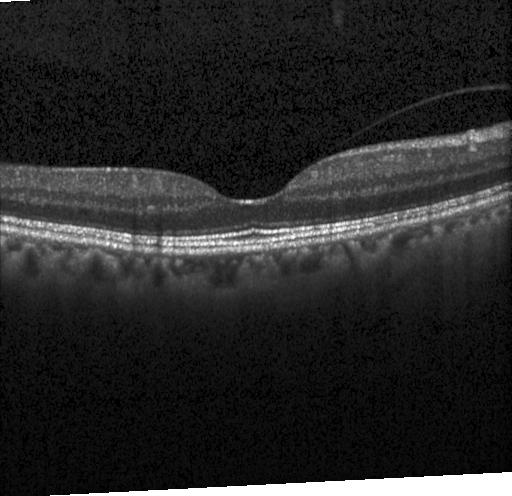

Diagnosis: neither CNV, DME, nor drusen.